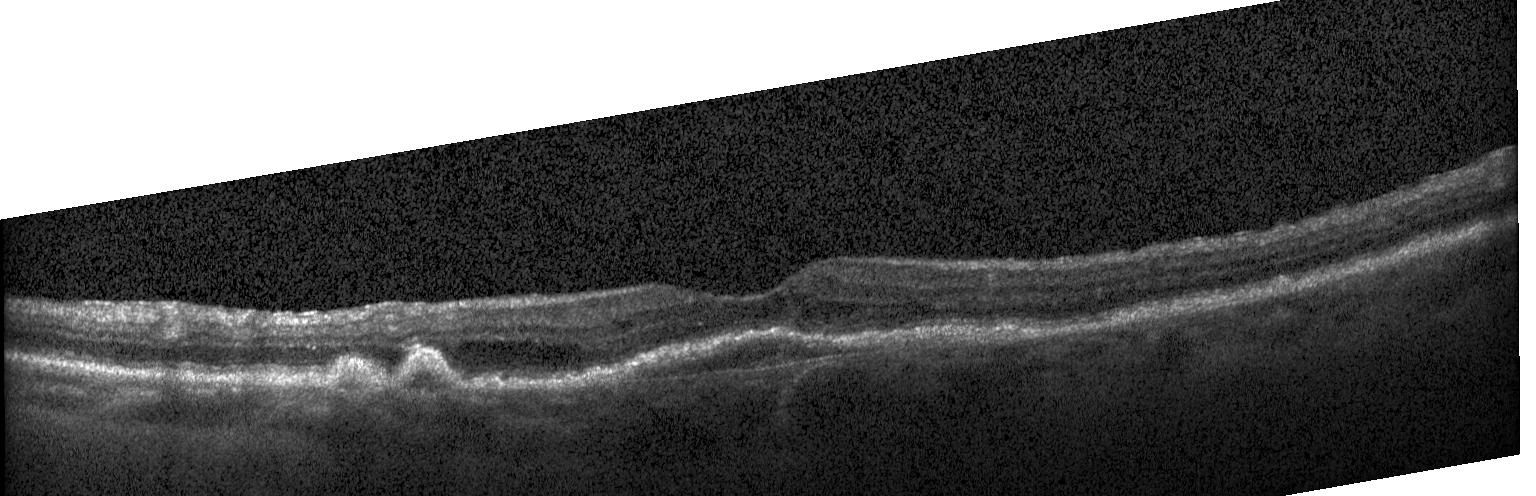
Diagnosis: a choroidal neovascular membrane.